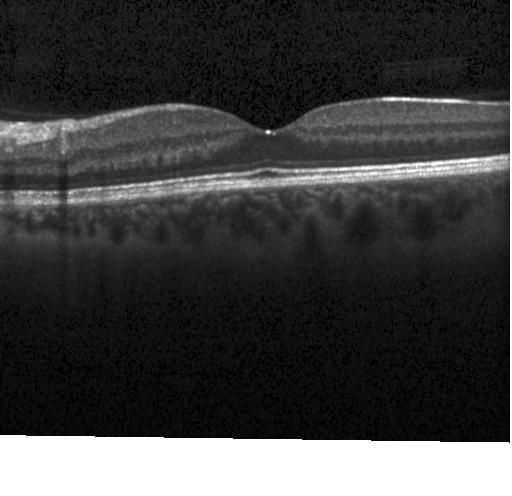
Macular OCT demonstrating no CNV, DME, or drusen.